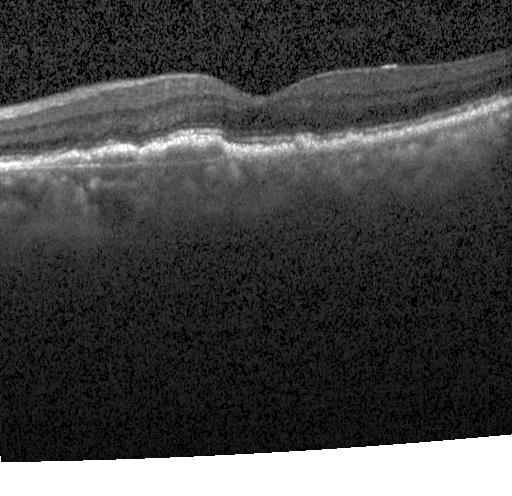
Centered on the fovea. Optical coherence tomography scan. Spectral-domain OCT. Impression: choroidal neovascularization (CNV).